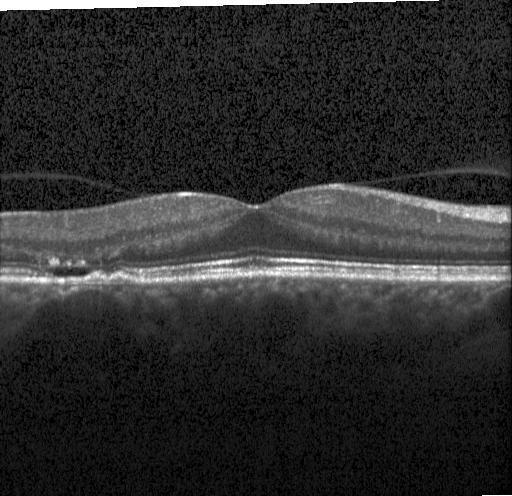 Spectral-domain optical coherence tomography · retinal OCT cross-section — Assessment: a choroidal neovascular membrane.